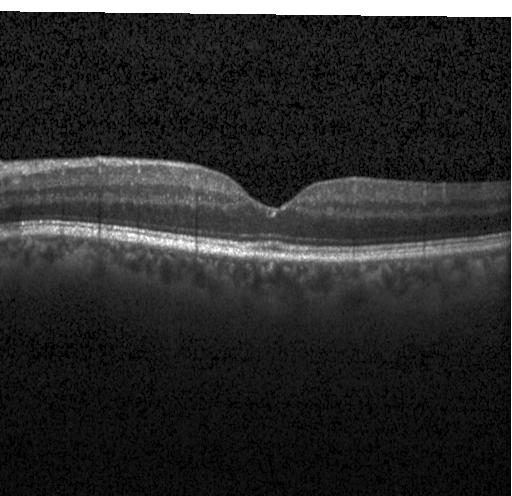 Retinal OCT B-scan · horizontal scan through the fovea — Impression: no choroidal neovascularization, diabetic macular edema, or drusen.